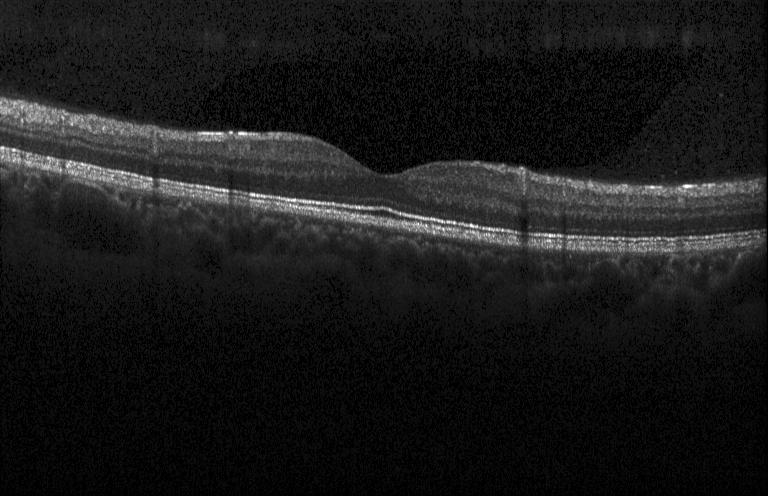 Retinal OCT B-scan · horizontal scan through the fovea — This B-scan demonstrates no choroidal neovascularization, diabetic macular edema, or drusen.